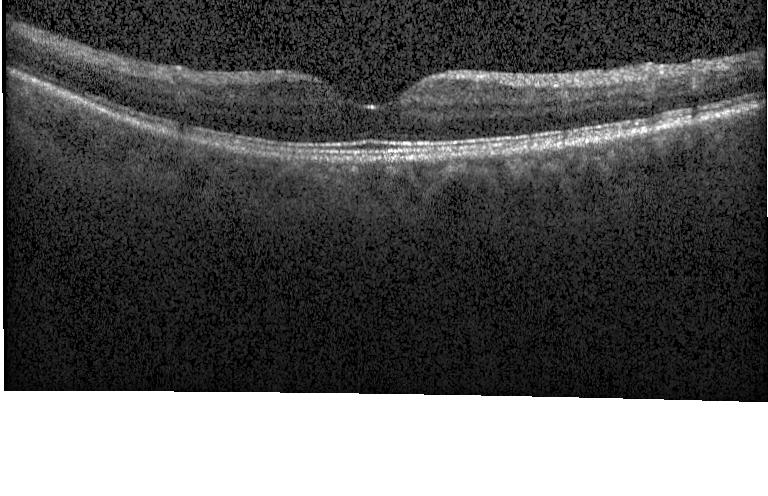
Instrument: Heidelberg Spectralis · retinal OCT cross-section
Impression: no choroidal neovascularization, diabetic macular edema, or drusen.